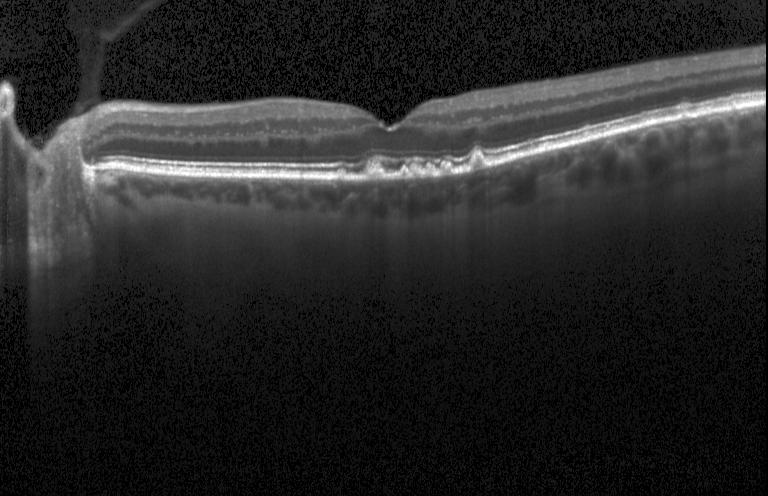 Dx: sub-RPE drusenoid deposits.